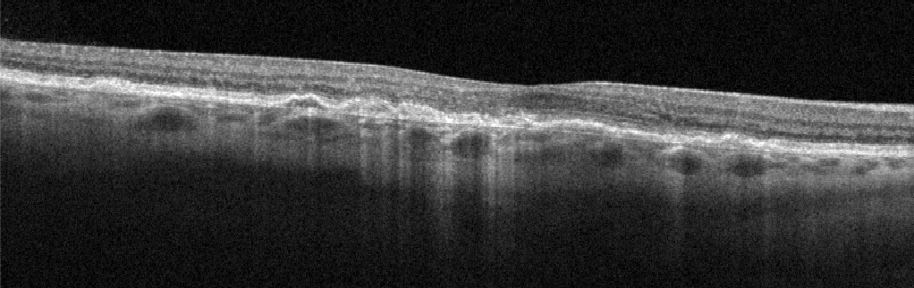
Finding: age-related macular degeneration (AMD).